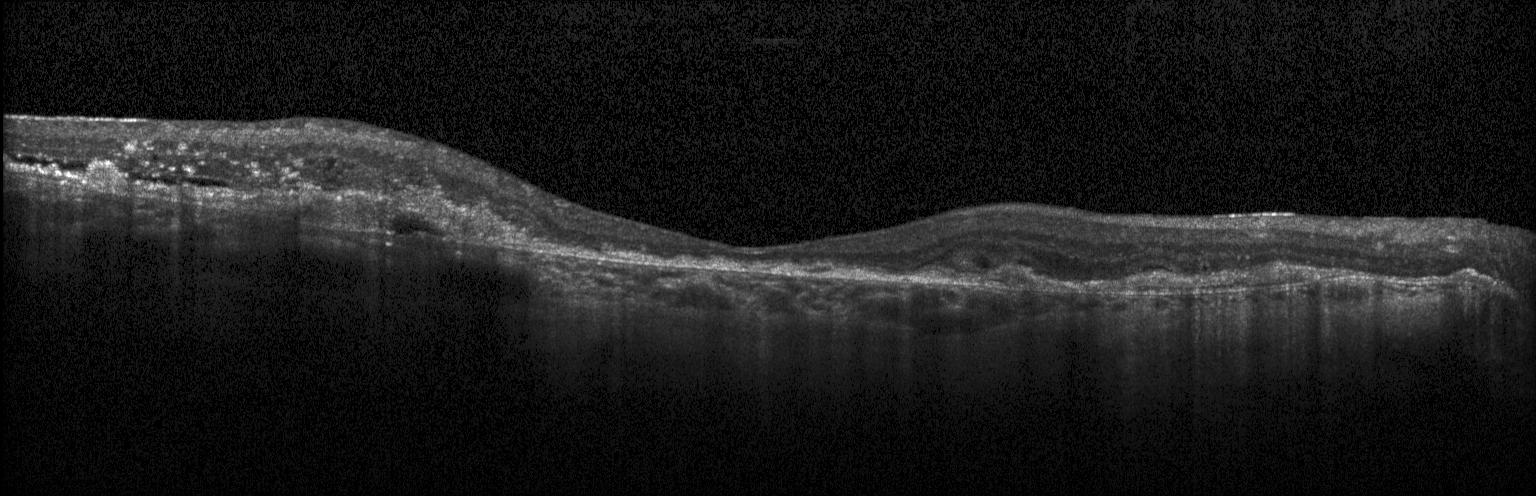
The scan shows choroidal neovascularization (CNV).